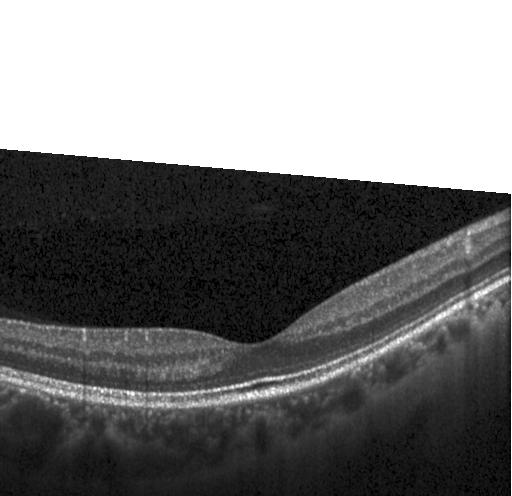
Spectral-domain optical coherence tomography; fovea-centered; optical coherence tomography B-scan — Impression: no choroidal neovascularization, no diabetic macular edema, and no drusen.